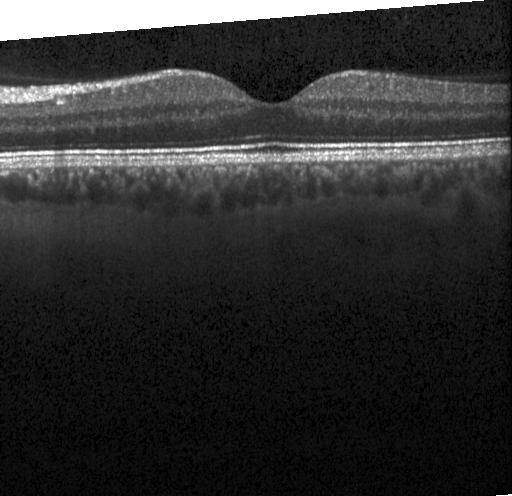 Assessment: no CNV, DME, or drusen.